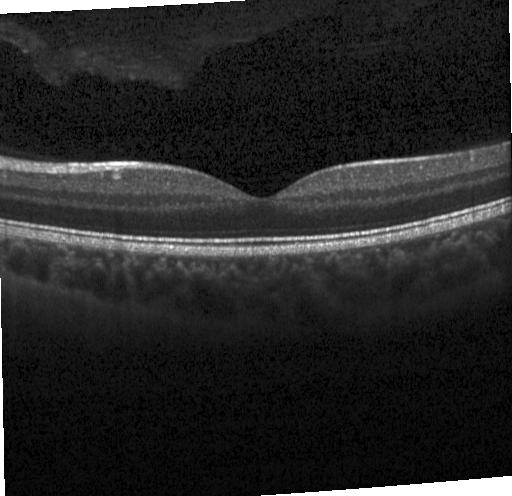 OCT B-scan · spectral-domain OCT.
Diagnosis: neither CNV, DME, nor drusen.